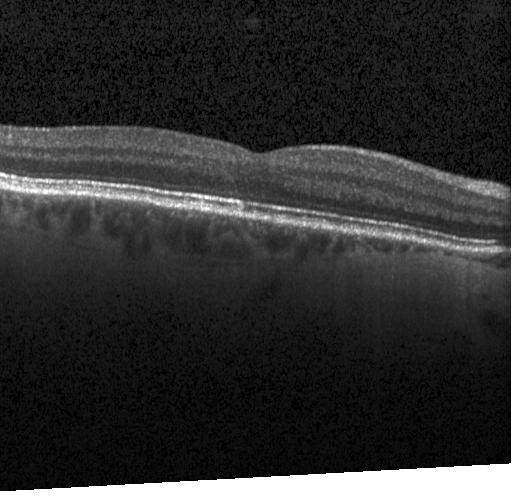 Optical coherence tomography B-scan. Spectral-domain optical coherence tomography.
Dx: no evidence of choroidal neovascularization, diabetic macular edema, or drusen.